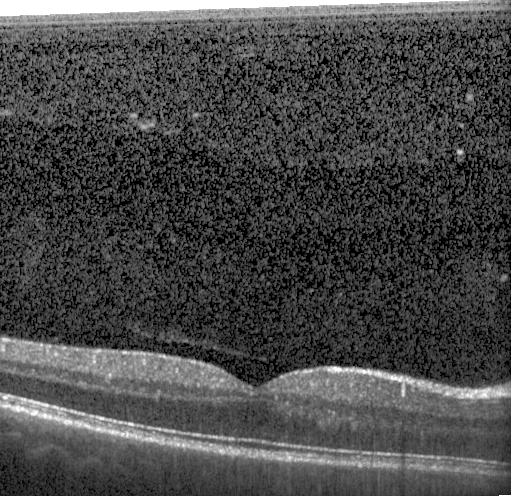
Retinal OCT cross-section. Through the macula. No choroidal neovascularization, no diabetic macular edema, and no drusen.